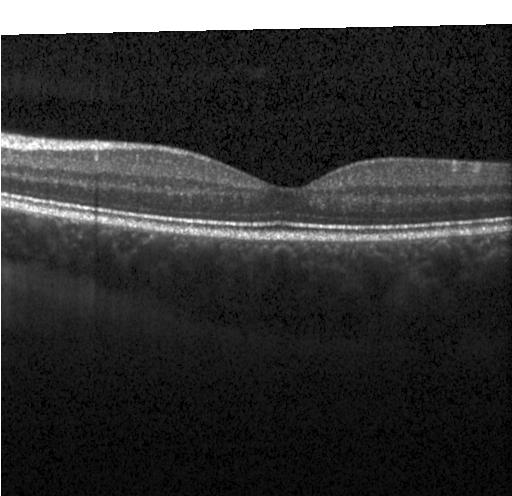 OCT B-scan · spectral-domain optical coherence tomography.
Diagnosis: no choroidal neovascularization, no diabetic macular edema, and no drusen.